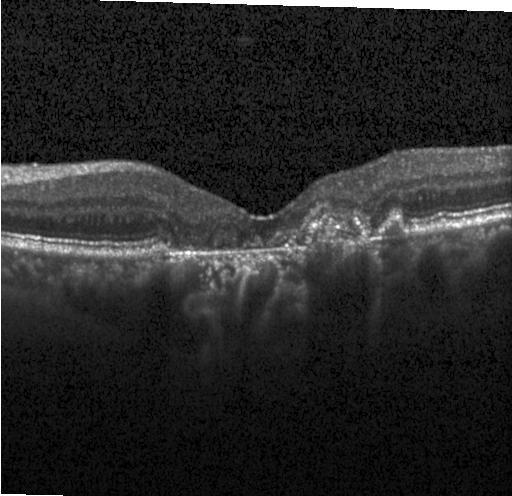

Macular scan, optical coherence tomography B-scan
Impression: CNV.